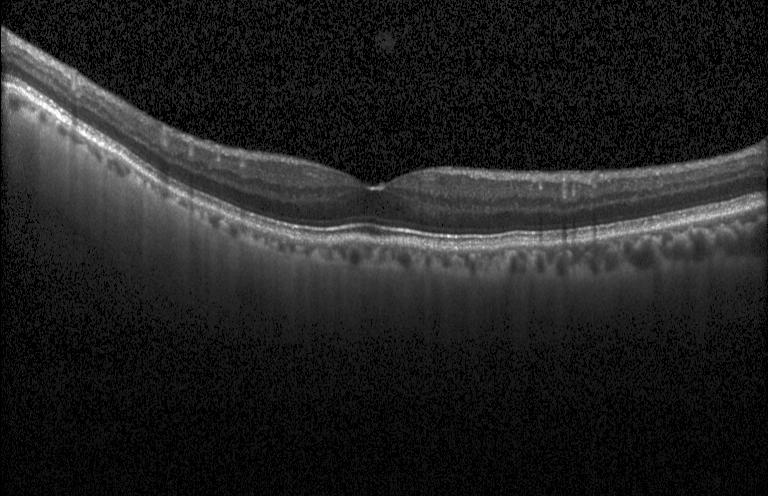

Optical coherence tomography B-scan, centered on the fovea, spectral-domain optical coherence tomography, instrument: Heidelberg Spectralis — OCT finding: no evidence of CNV, DME, or drusen.